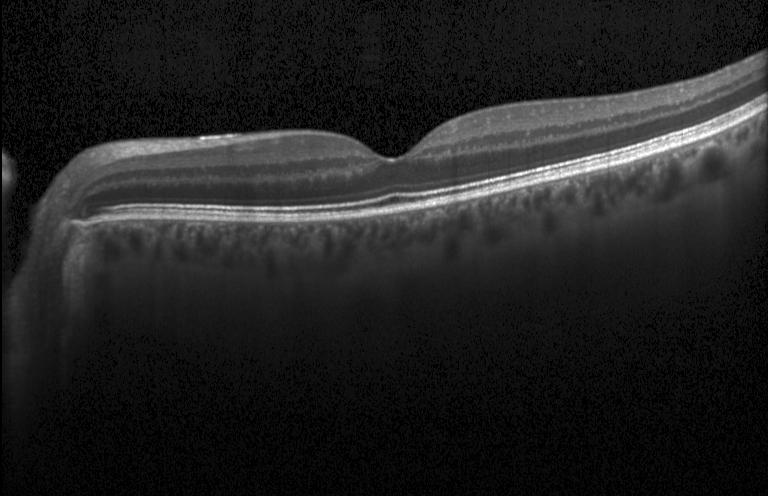
Macular scan, SD-OCT, retinal OCT B-scan, acquired on a Heidelberg Spectralis. Diagnosis: neither choroidal neovascularization, diabetic macular edema, nor drusen.